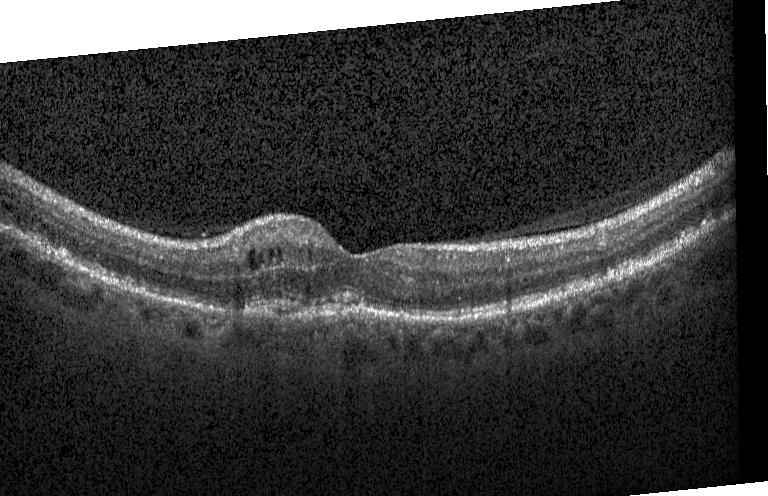 Retinal OCT cross-section showing a choroidal neovascular membrane.